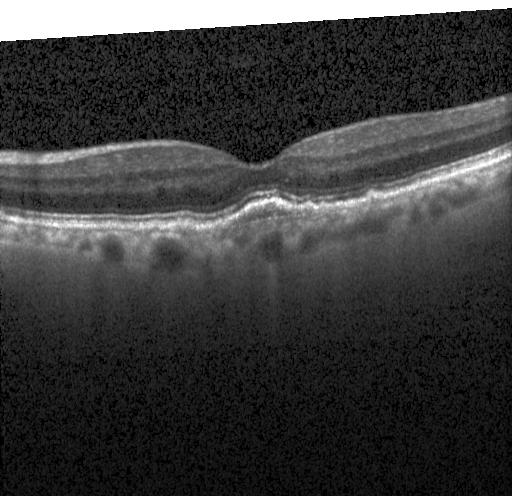 Optical coherence tomography scan, Heidelberg Spectralis, spectral-domain OCT.
Macular OCT: a choroidal neovascular membrane.